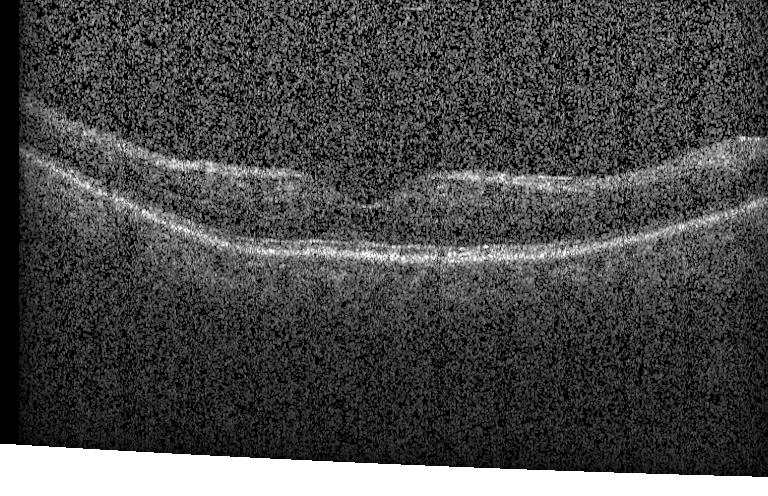
This B-scan demonstrates neither choroidal neovascularization, diabetic macular edema, nor drusen.